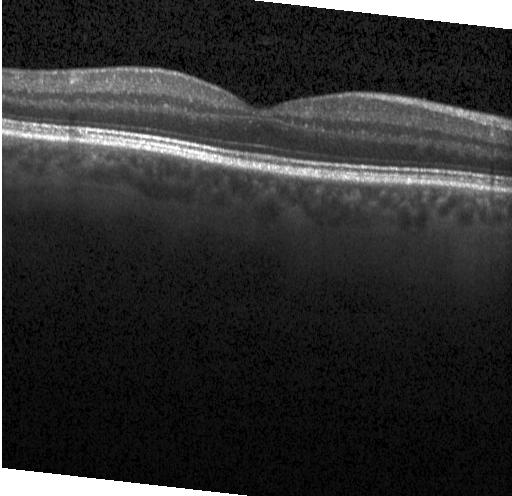 The scan shows no CNV, no DME, and no drusen.